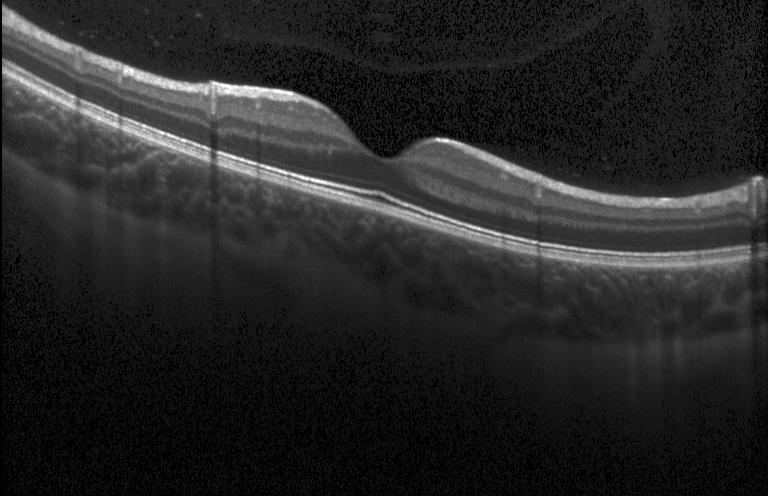 Finding: neither choroidal neovascularization, diabetic macular edema, nor drusen.